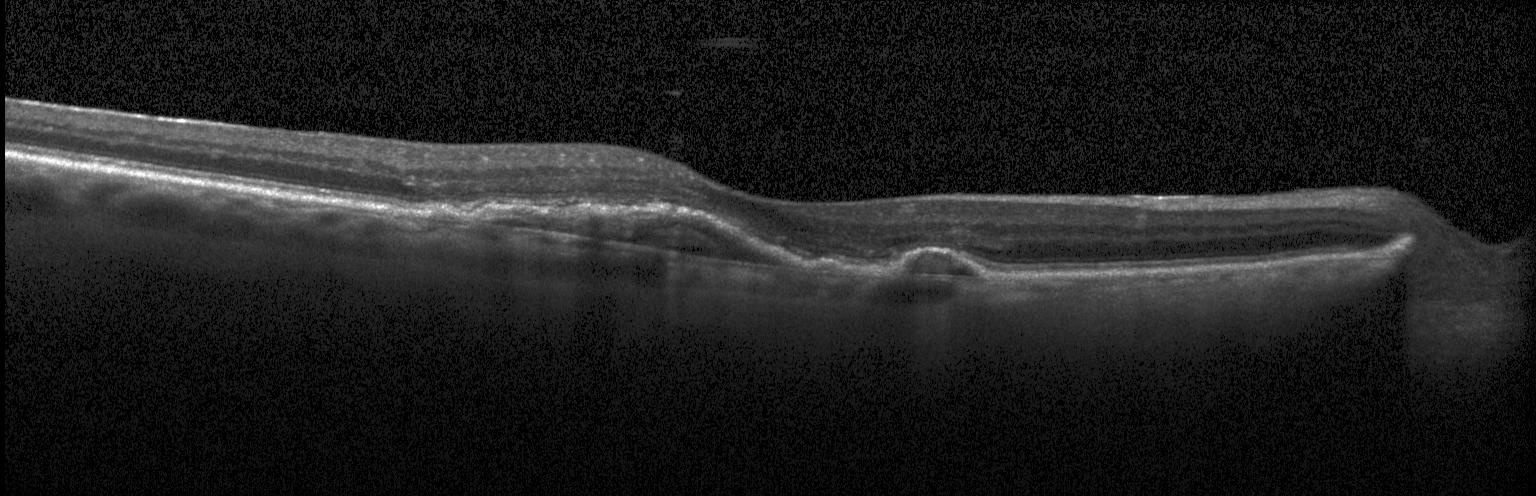 Spectral-domain optical coherence tomography; Heidelberg Spectralis; retinal OCT B-scan; horizontal scan through the fovea
Diagnosis: choroidal neovascularization.